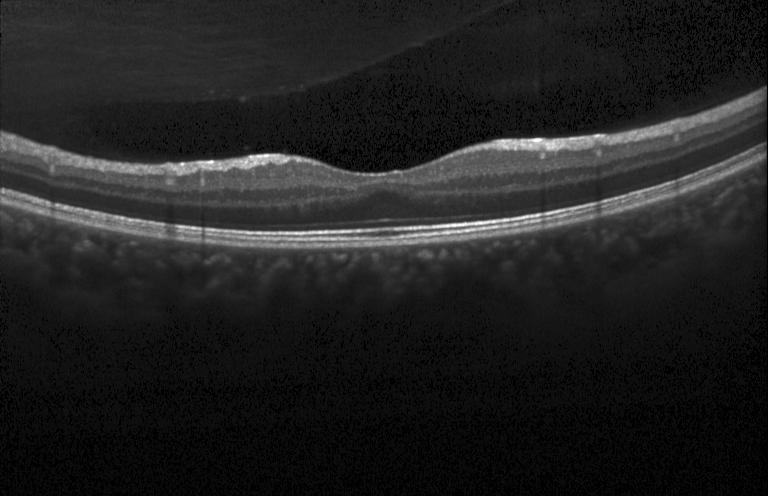 OCT B-scan. Macular OCT: neither choroidal neovascularization, diabetic macular edema, nor drusen.